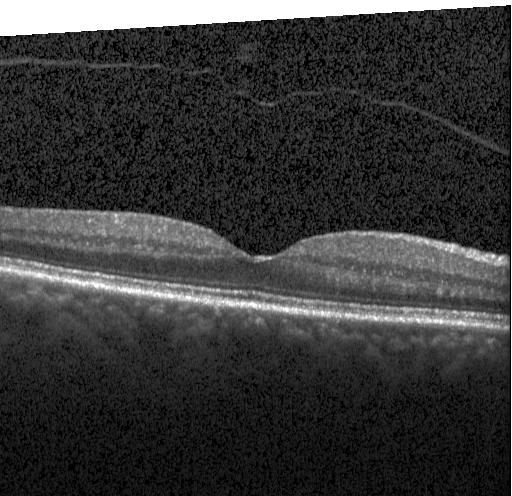
Retinal OCT cross-section; Heidelberg Spectralis OCT system; through the macula — Macular OCT: no choroidal neovascularization, diabetic macular edema, or drusen.